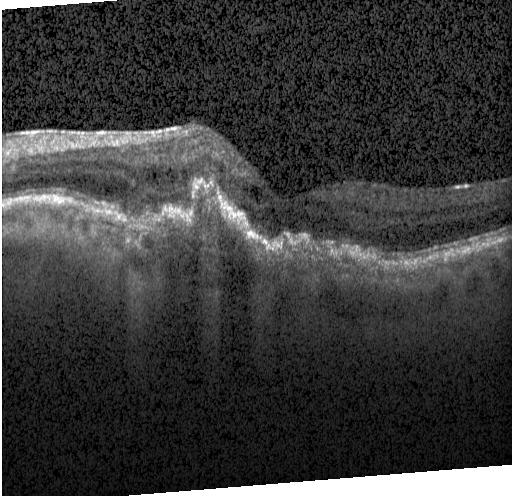

Retinal OCT B-scan, spectral-domain optical coherence tomography, acquired on a Heidelberg Spectralis.
Impression: choroidal neovascularization (CNV).